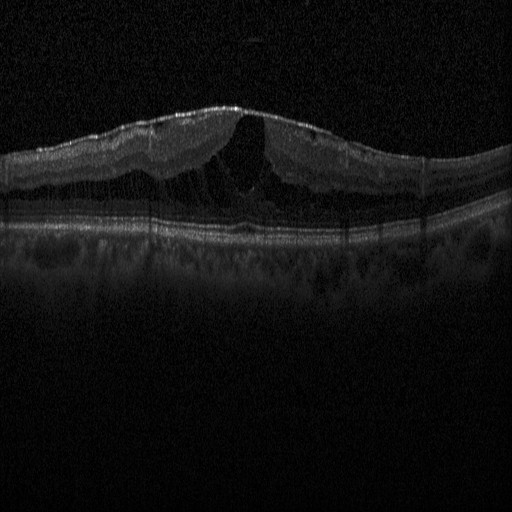

OCT line scan. Spectral-domain OCT. Through the macula. Heidelberg Spectralis
OCT finding: diabetic macular edema.